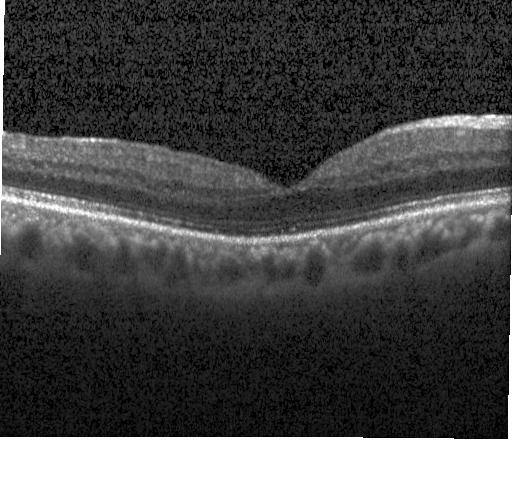
OCT B-scan
Diagnosis: no CNV, no DME, and no drusen.